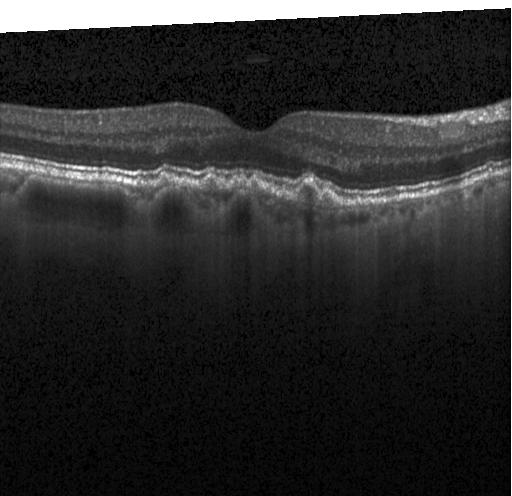
OCT B-scan; fovea-centered — Finding: drusen.